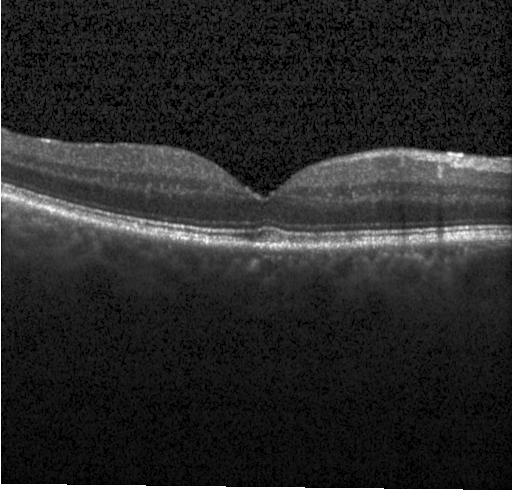

This B-scan demonstrates no CNV, DME, or drusen.